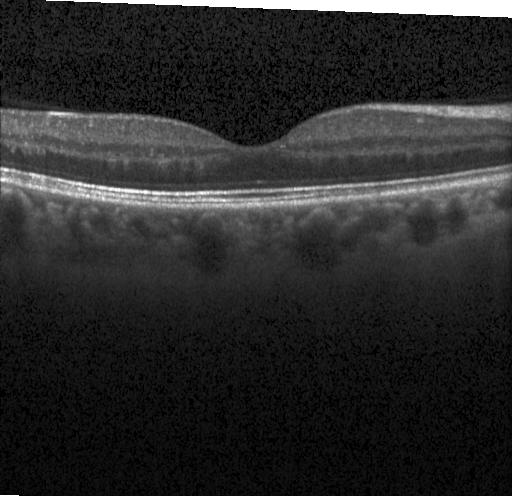 SD-OCT, OCT line scan, Heidelberg Spectralis.
Diagnosis: no choroidal neovascularization, no diabetic macular edema, and no drusen.